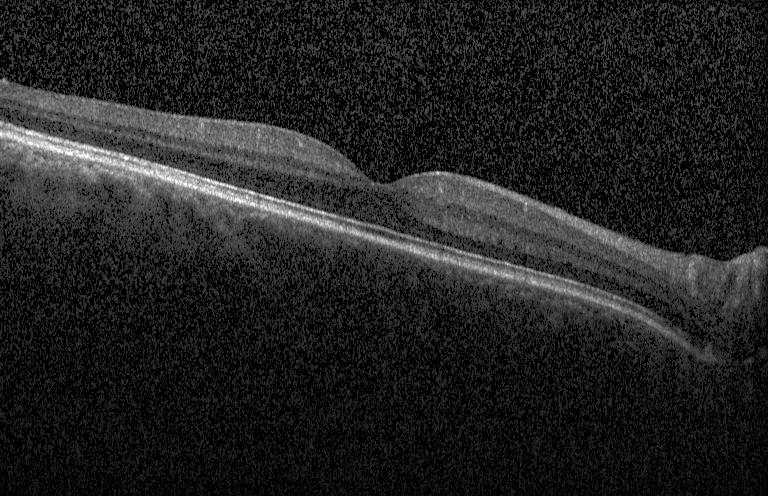
Diagnosis: no CNV, DME, or drusen.